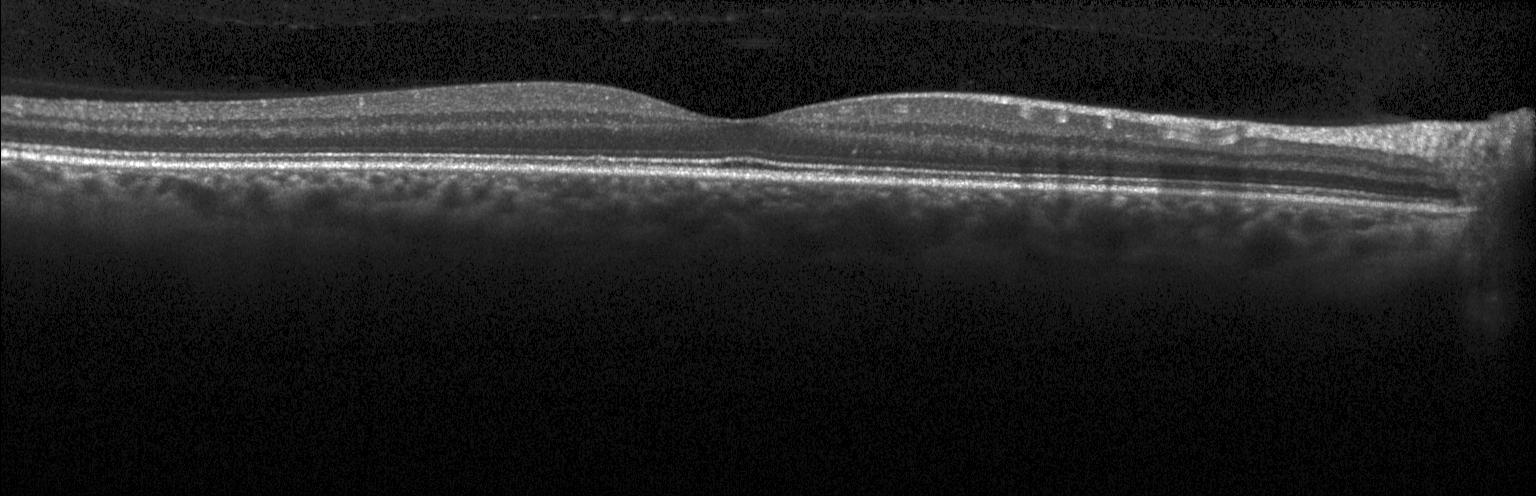 OCT B-scan showing no evidence of CNV, DME, or drusen.